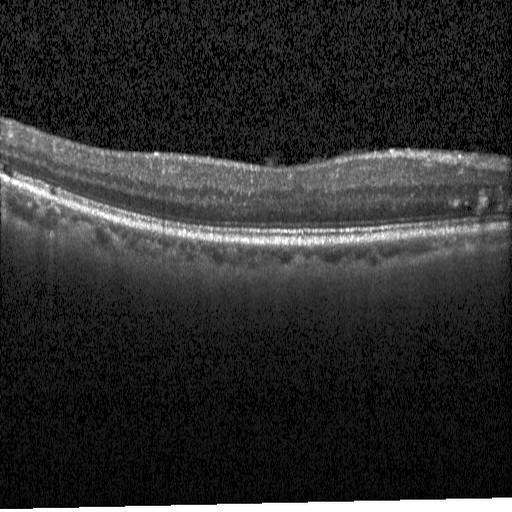

OCT line scan · Heidelberg Spectralis OCT system · spectral-domain optical coherence tomography.
The scan shows diabetic macular edema (DME).